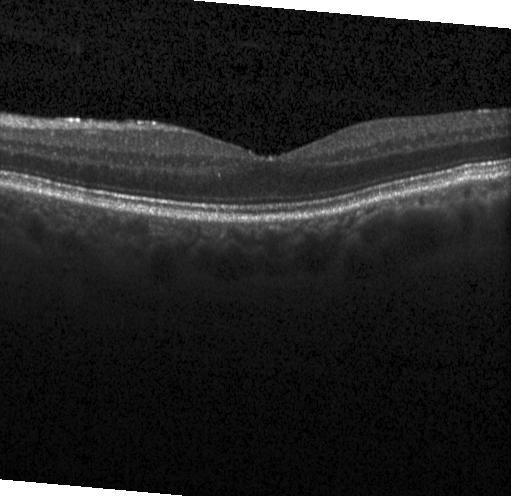 OCT B-scan showing no choroidal neovascularization, diabetic macular edema, or drusen.